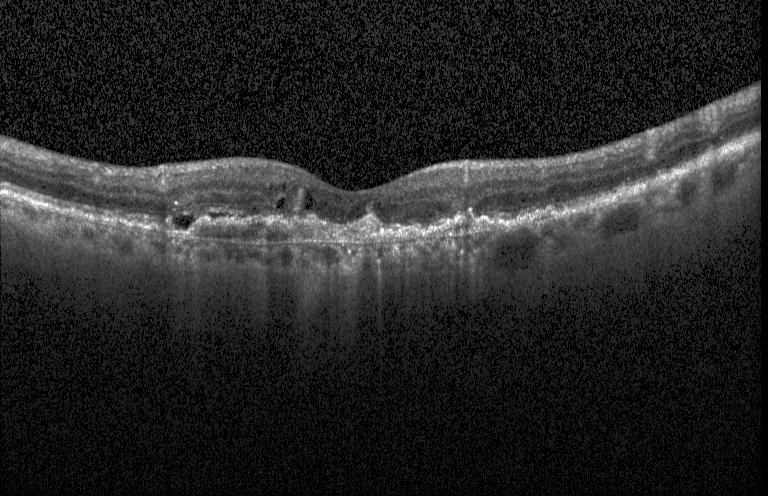 OCT line scan — Finding: a choroidal neovascular membrane.